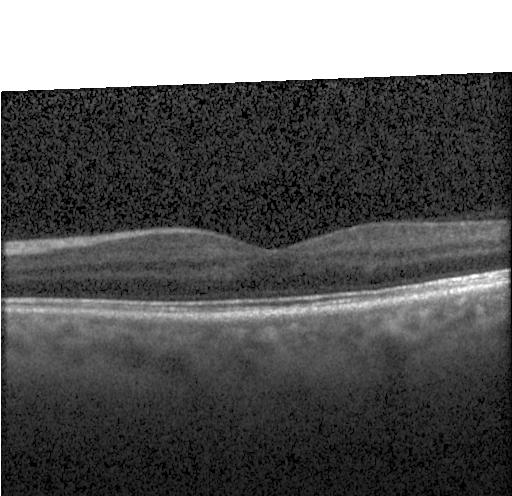
Finding: no CNV, DME, or drusen.